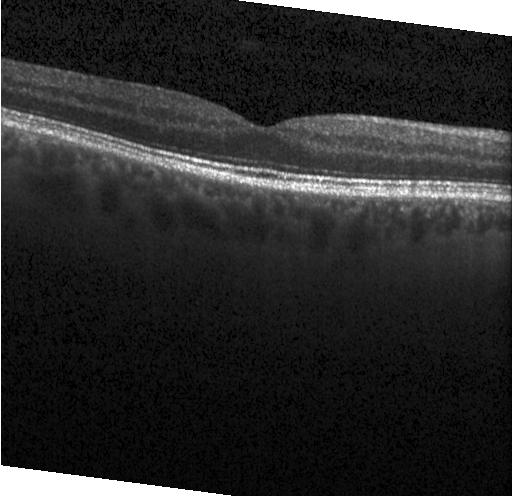
Retinal OCT cross-section, spectral-domain OCT. Impression: no evidence of choroidal neovascularization, diabetic macular edema, or drusen.